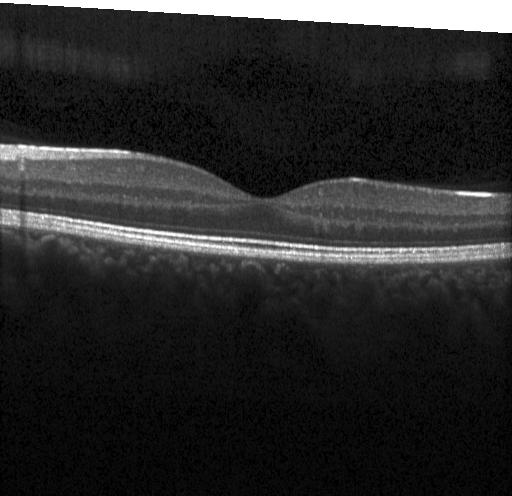

Retinal OCT B-scan
Finding: no evidence of choroidal neovascularization, diabetic macular edema, or drusen.